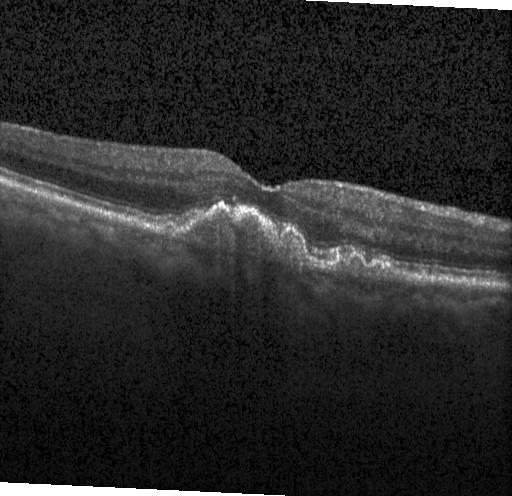
Optical coherence tomography scan.
OCT finding: a choroidal neovascular membrane.